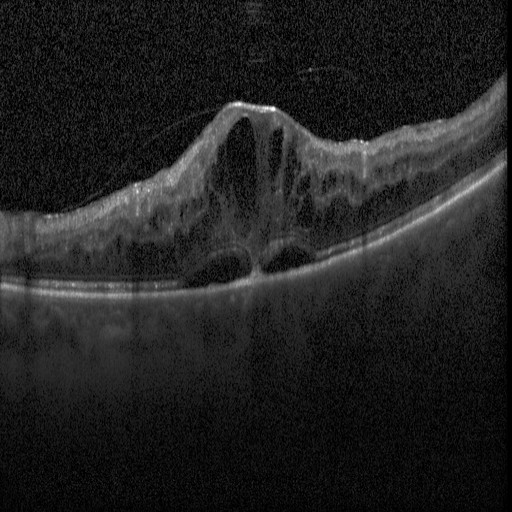 Spectral-domain OCT B-scan: DME.